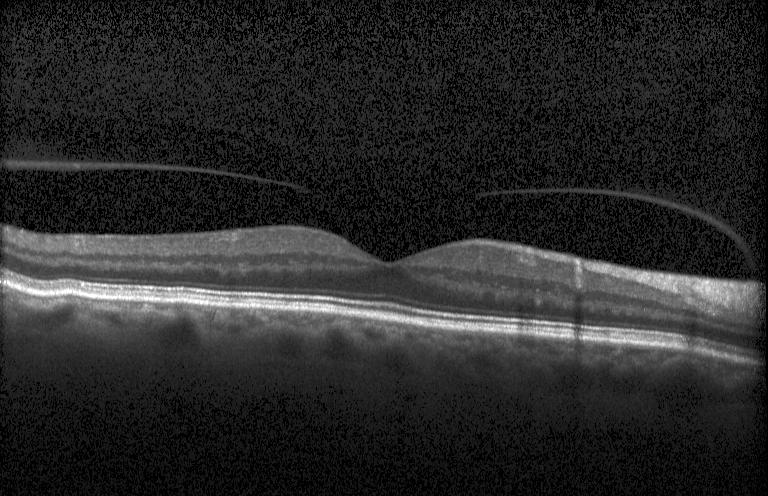

OCT B-scan — Impression: neither choroidal neovascularization, diabetic macular edema, nor drusen.